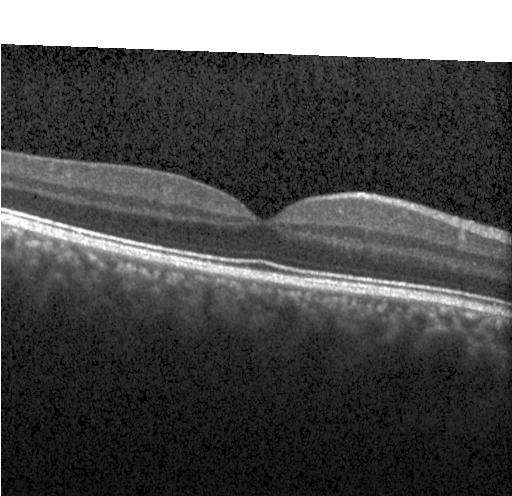 Retinal OCT B-scan, SD-OCT, fovea-centered
Diagnosis: no choroidal neovascularization, no diabetic macular edema, and no drusen.